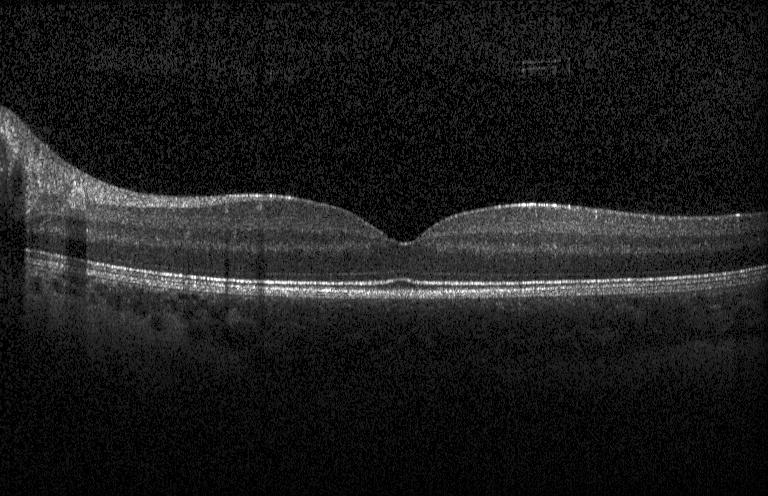
No CNV, no DME, and no drusen.